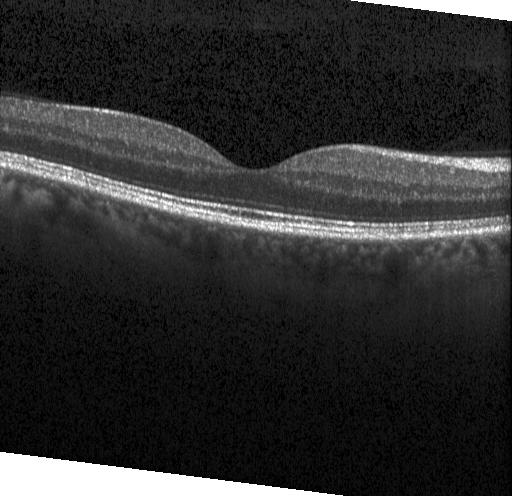

Centered on the fovea, acquired on a Heidelberg Spectralis, spectral-domain OCT, optical coherence tomography scan — Impression: no CNV, DME, or drusen.